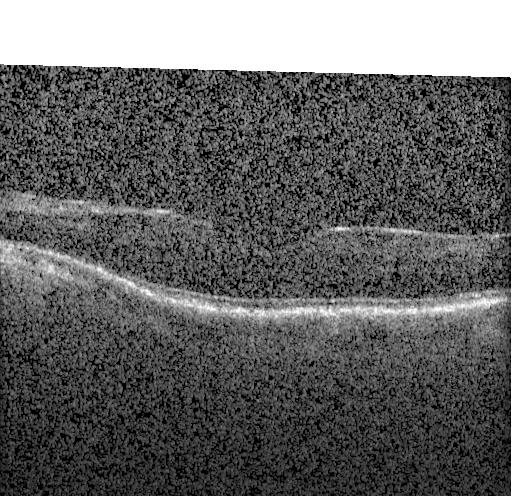 Finding: no choroidal neovascularization, diabetic macular edema, or drusen.